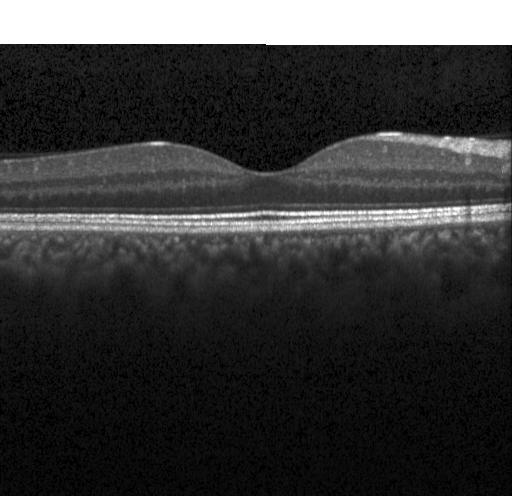

Macular OCT demonstrating no evidence of CNV, DME, or drusen.